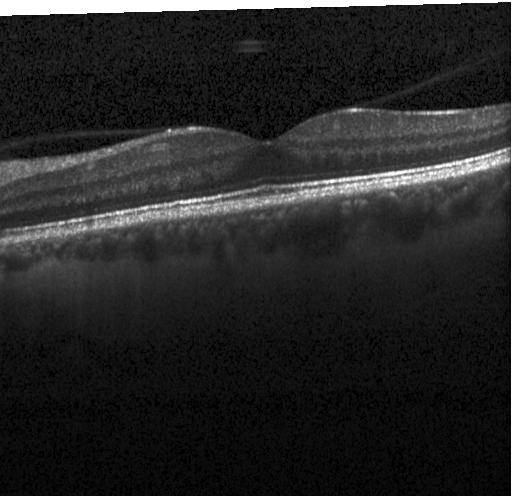 Spectral-domain OCT B-scan: no choroidal neovascularization, no diabetic macular edema, and no drusen.